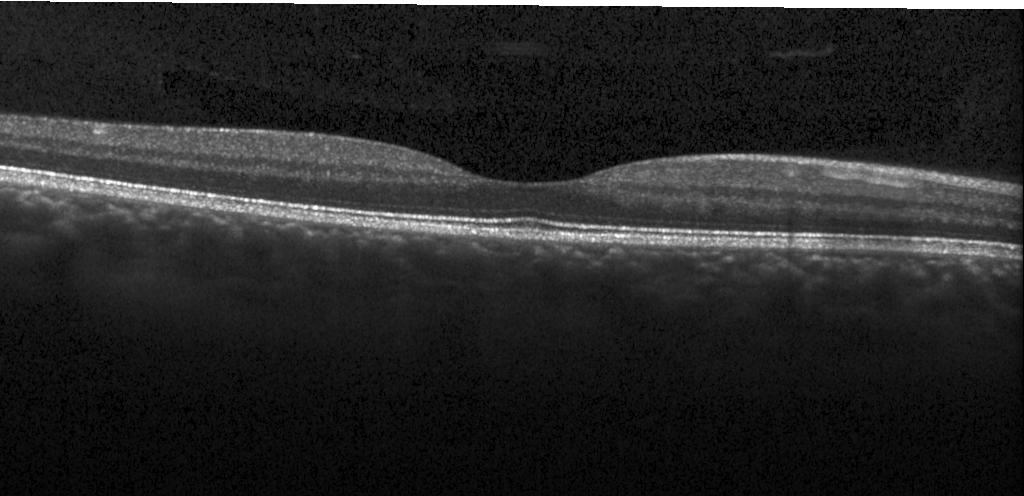

Impression: neither CNV, DME, nor drusen.